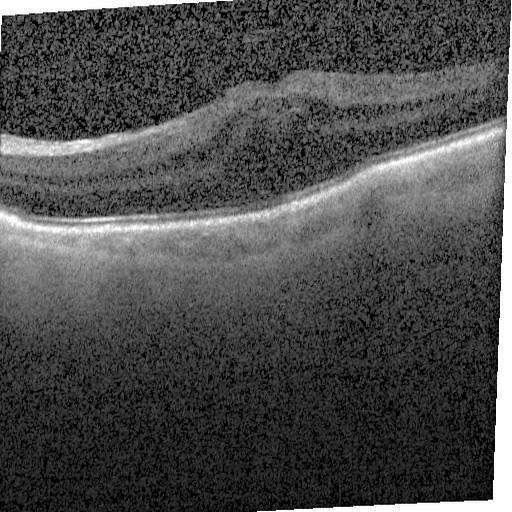

Instrument: Heidelberg Spectralis · retinal OCT B-scan. Impression: DME.